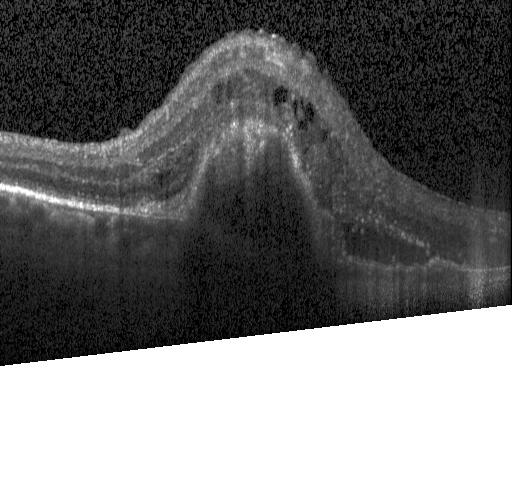 Retinal OCT B-scan, Heidelberg Spectralis OCT system. The scan shows choroidal neovascularization (CNV).